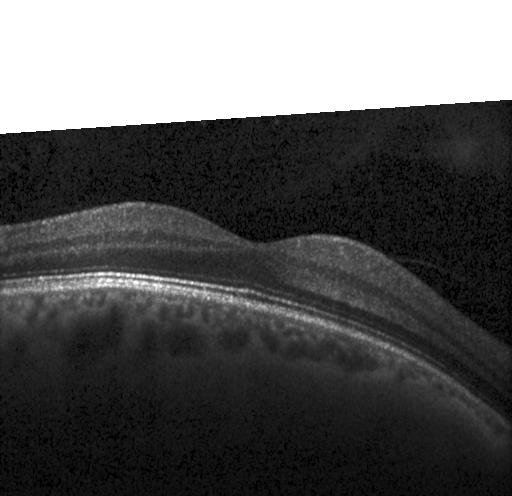
Impression: no choroidal neovascularization, no diabetic macular edema, and no drusen.